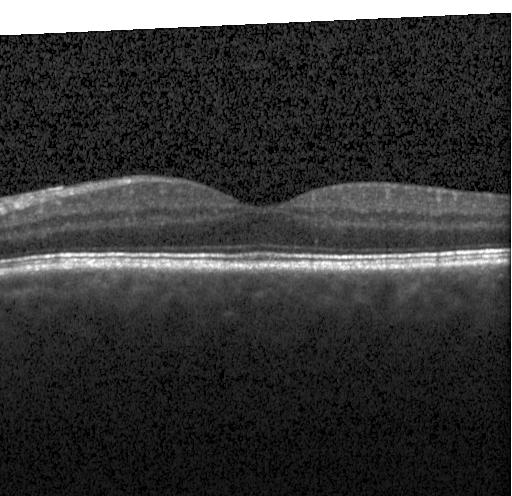
Optical coherence tomography B-scan, acquired on a Heidelberg Spectralis, spectral-domain OCT.
Diagnosis: no evidence of CNV, DME, or drusen.